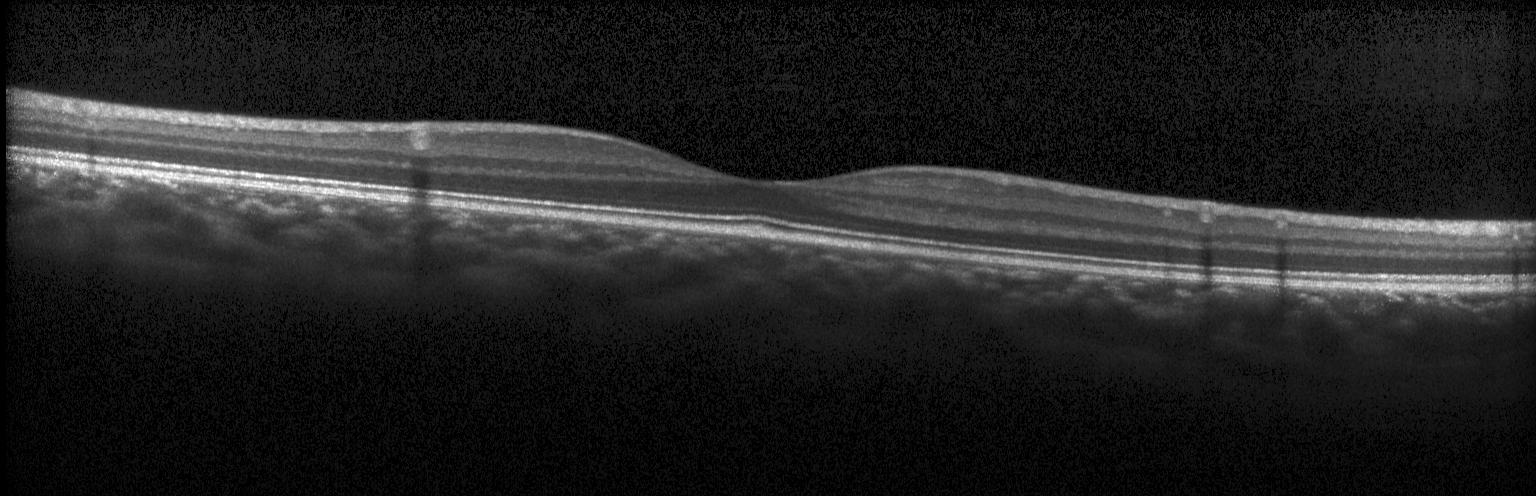 Heidelberg Spectralis, optical coherence tomography scan, spectral-domain OCT, horizontal scan through the fovea — OCT finding: neither choroidal neovascularization, diabetic macular edema, nor drusen.